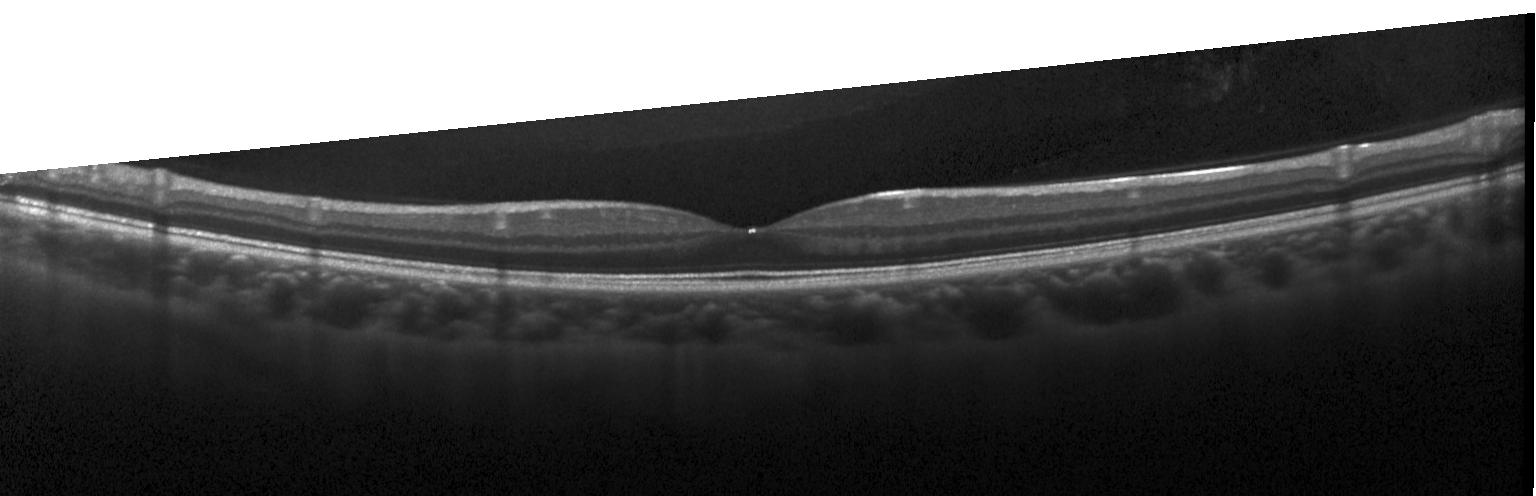

Impression: no CNV, no DME, and no drusen.